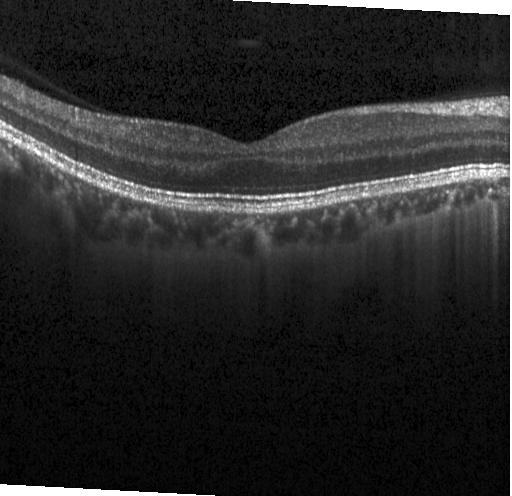 Impression: no choroidal neovascularization, diabetic macular edema, or drusen.